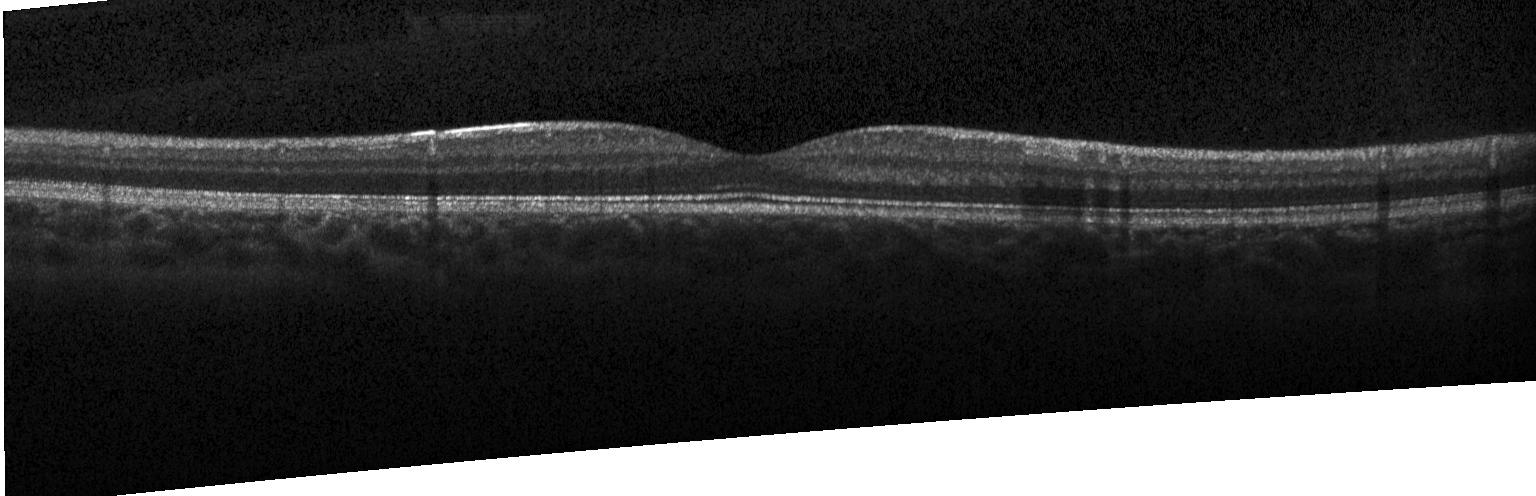

Optical coherence tomography scan — Dx: no evidence of choroidal neovascularization, diabetic macular edema, or drusen.